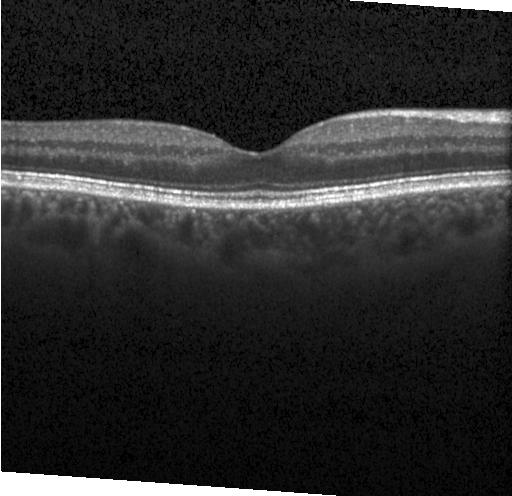

Retinal OCT cross-section showing no choroidal neovascularization, diabetic macular edema, or drusen.